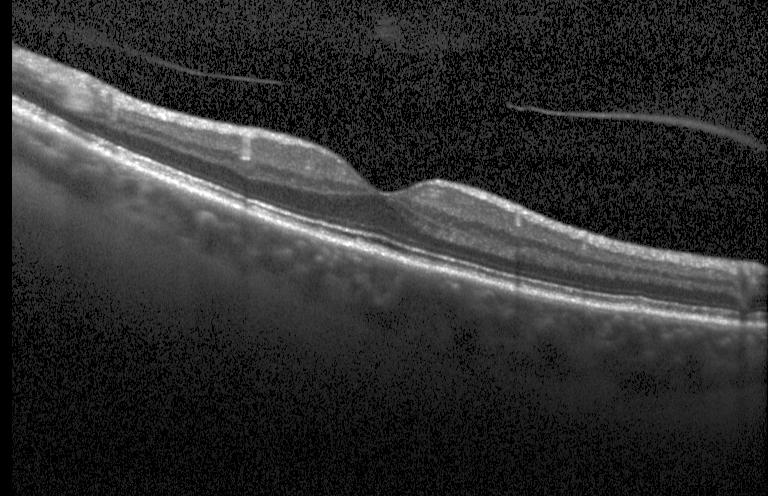
OCT line scan — Impression: no choroidal neovascularization, no diabetic macular edema, and no drusen.